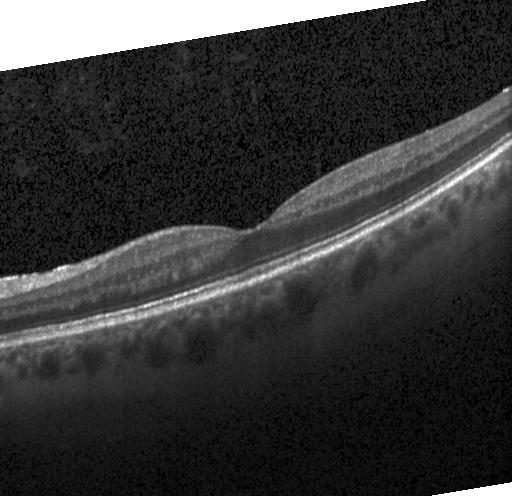

Retinal OCT cross-section. No CNV, DME, or drusen.